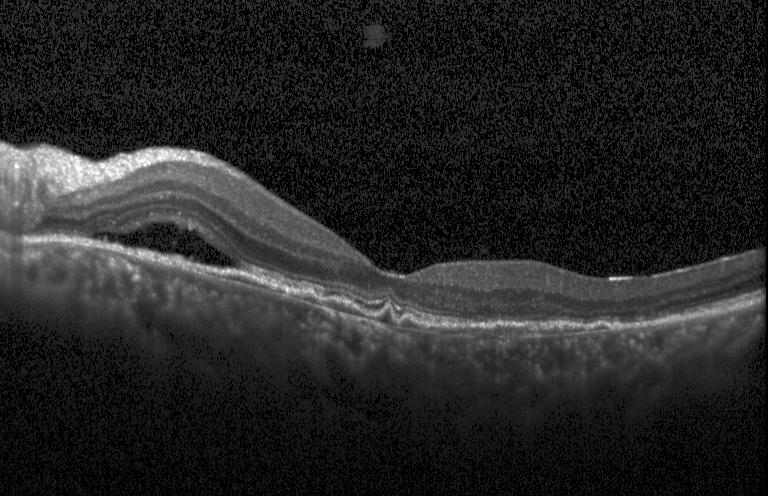

Choroidal neovascularization (CNV).